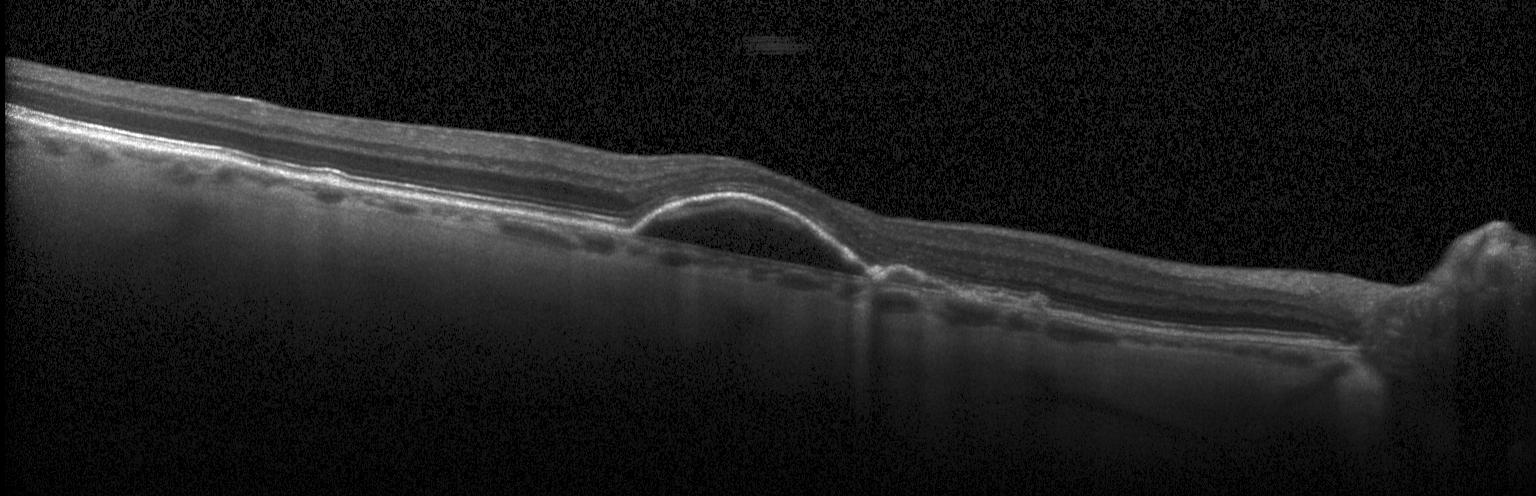

Impression: a choroidal neovascular membrane.